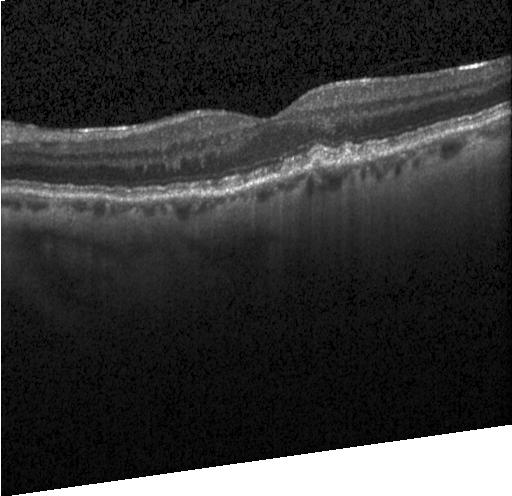 OCT line scan — The scan shows drusen.